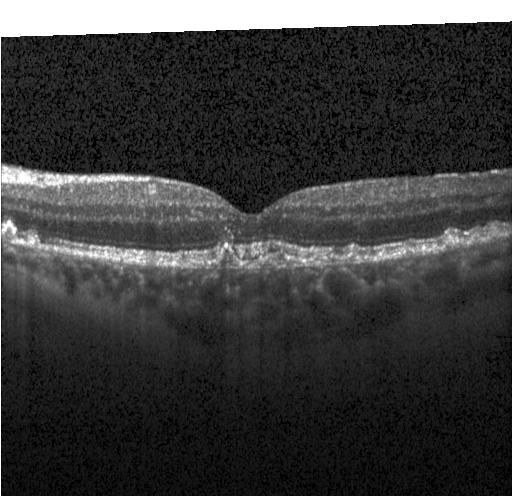

Heidelberg Spectralis · OCT line scan
Diagnosis: CNV.